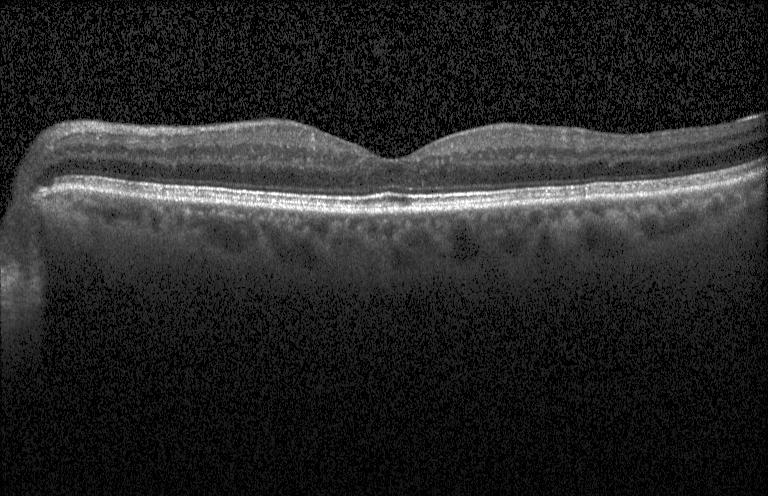

OCT B-scan, spectral-domain optical coherence tomography, horizontal scan through the fovea. Dx: neither CNV, DME, nor drusen.